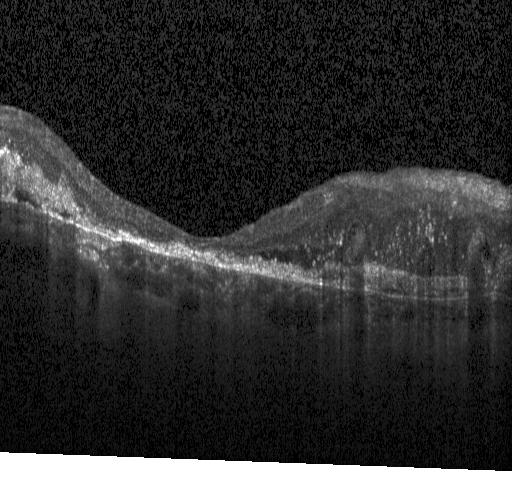
The scan shows choroidal neovascularization.